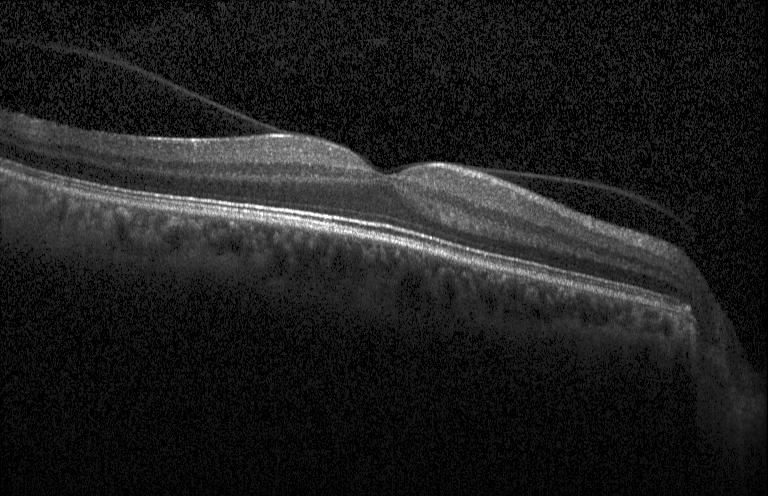

Heidelberg Spectralis OCT system, optical coherence tomography scan.
Finding: no CNV, DME, or drusen.